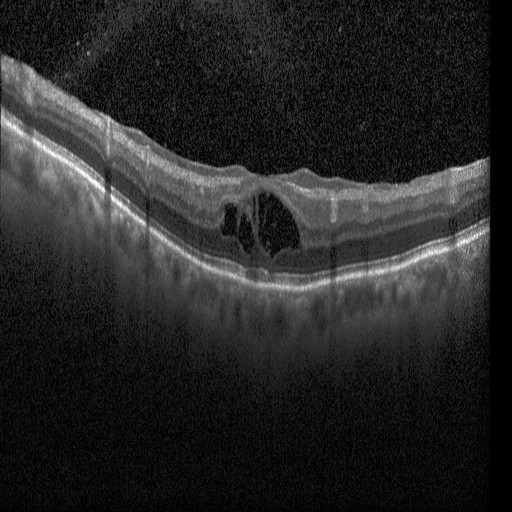 Heidelberg Spectralis OCT system · optical coherence tomography scan · horizontal scan through the fovea — Diagnosis: DME.